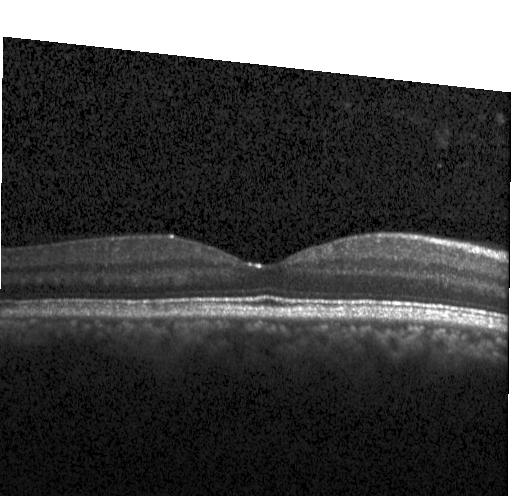
Retinal OCT cross-section showing neither CNV, DME, nor drusen.